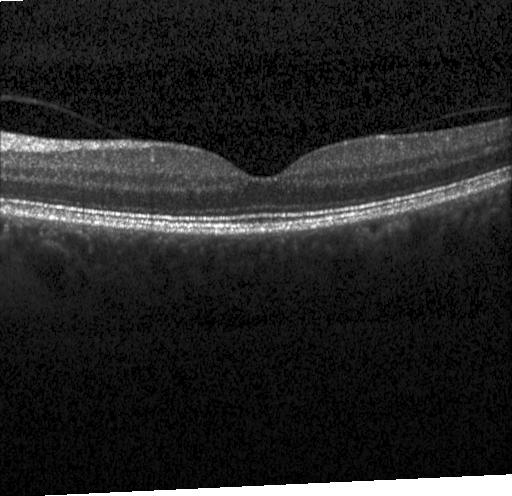 Retinal OCT cross-section — Finding: no choroidal neovascularization, diabetic macular edema, or drusen.